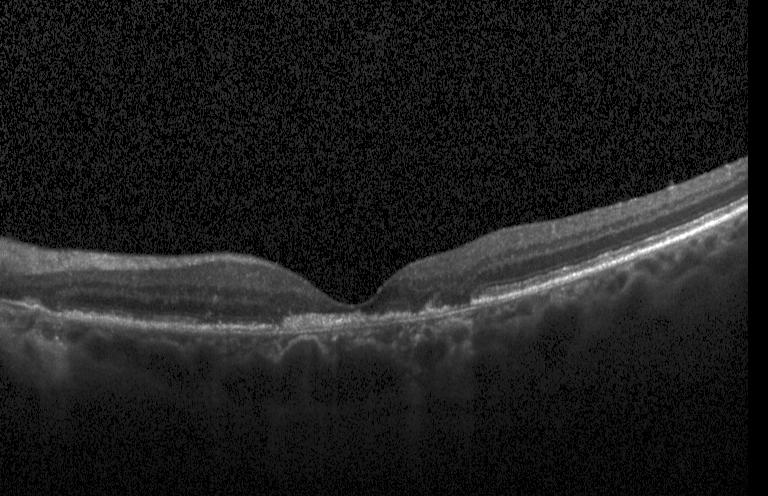
OCT B-scan. Impression: CNV.